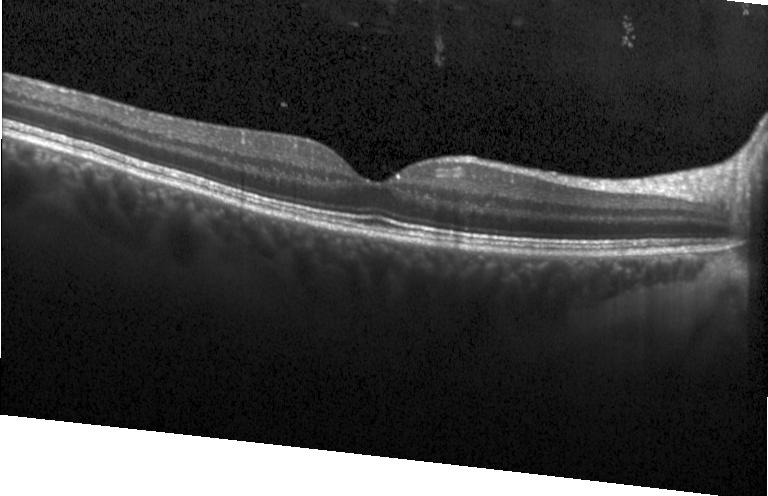 Acquired on a Heidelberg Spectralis, optical coherence tomography B-scan.
Impression: no choroidal neovascularization, diabetic macular edema, or drusen.